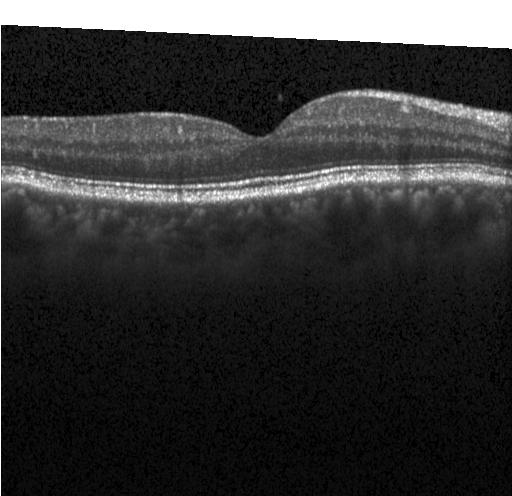
Spectral-domain OCT; OCT B-scan; acquired on a Heidelberg Spectralis; through the macula
No evidence of choroidal neovascularization, diabetic macular edema, or drusen.